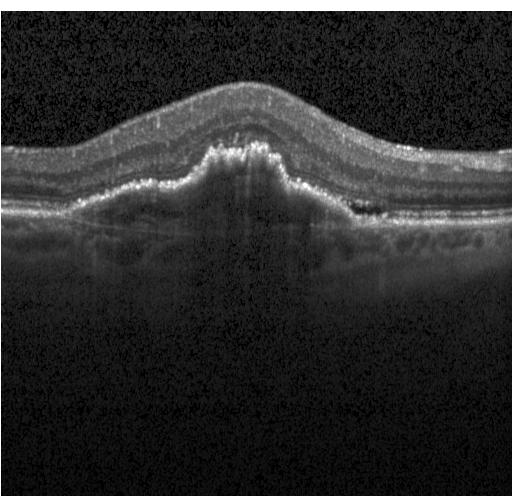
Finding: CNV.